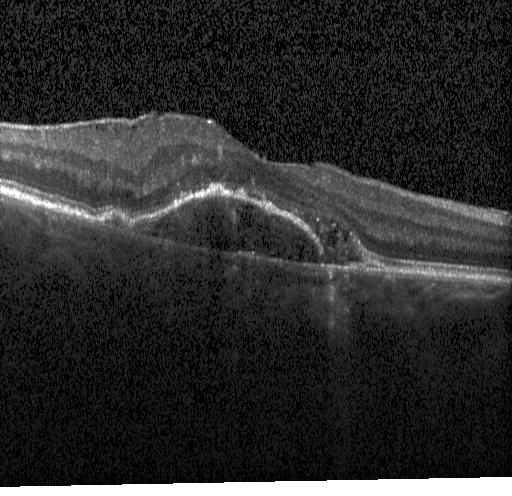
Retinal OCT cross-section showing a choroidal neovascular membrane.